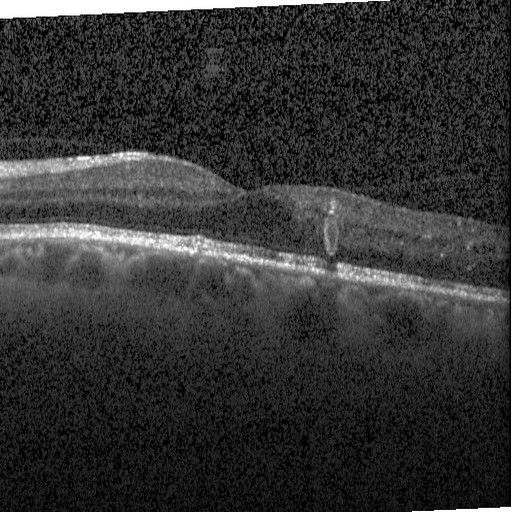 OCT line scan, spectral-domain optical coherence tomography, macular scan, Heidelberg Spectralis — Diagnosis: DME.